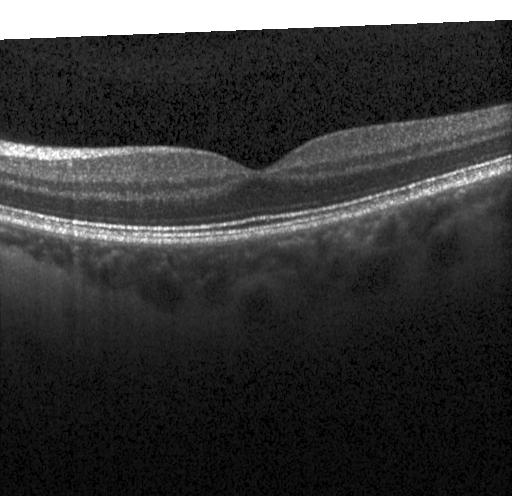

Macular scan · retinal OCT B-scan.
Impression: neither choroidal neovascularization, diabetic macular edema, nor drusen.